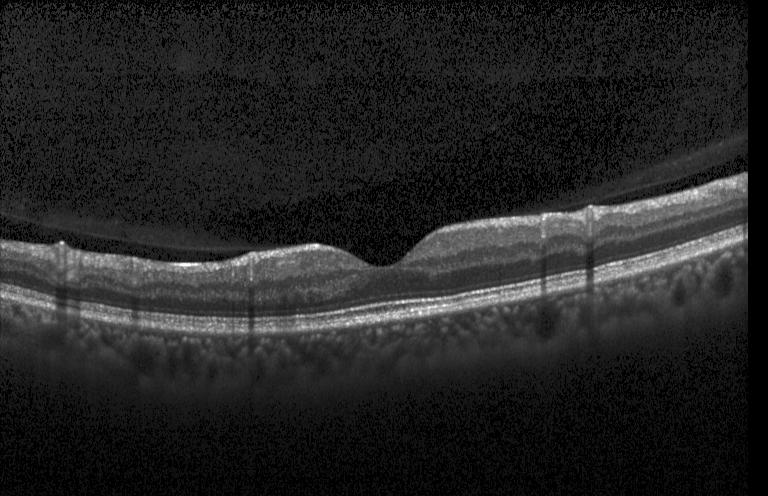
Diagnosis: neither choroidal neovascularization, diabetic macular edema, nor drusen.